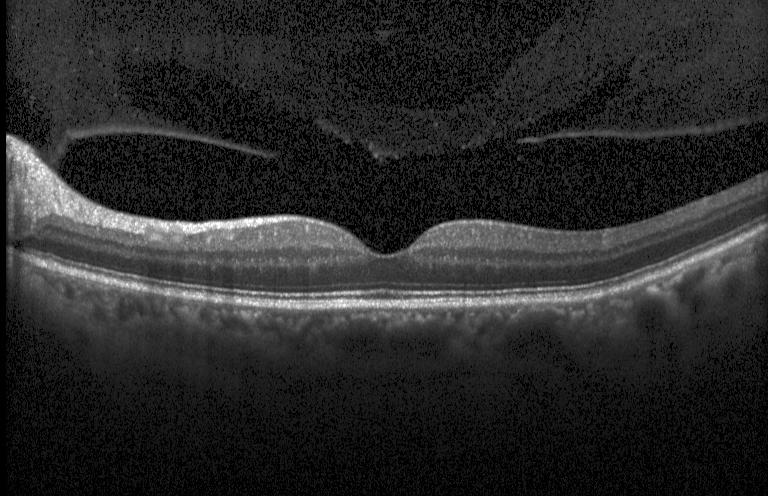 This B-scan demonstrates neither CNV, DME, nor drusen.